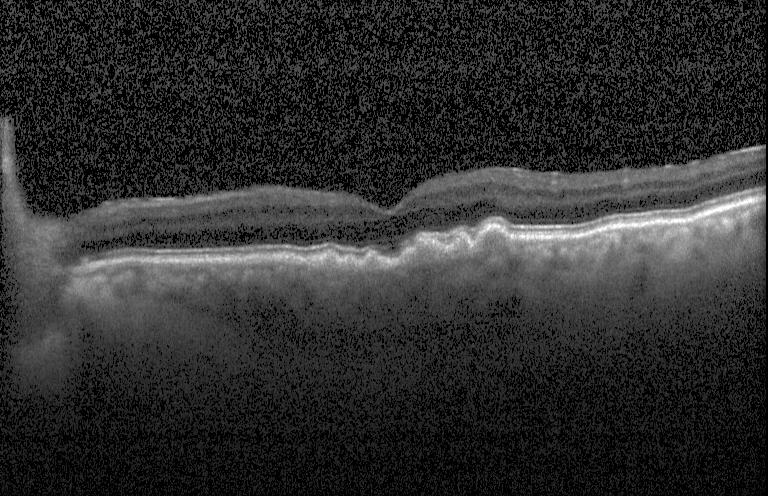
This B-scan demonstrates sub-RPE drusenoid deposits.